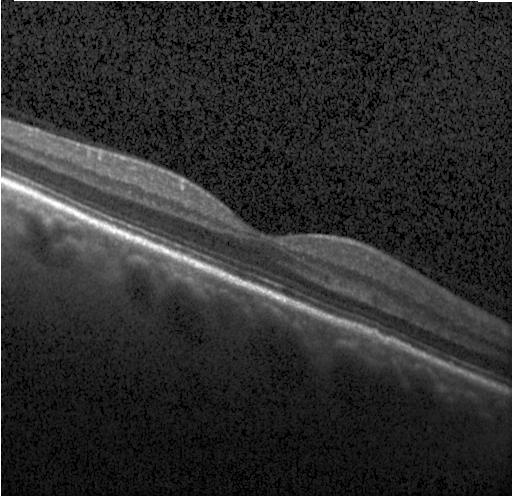 Assessment: no CNV, DME, or drusen.